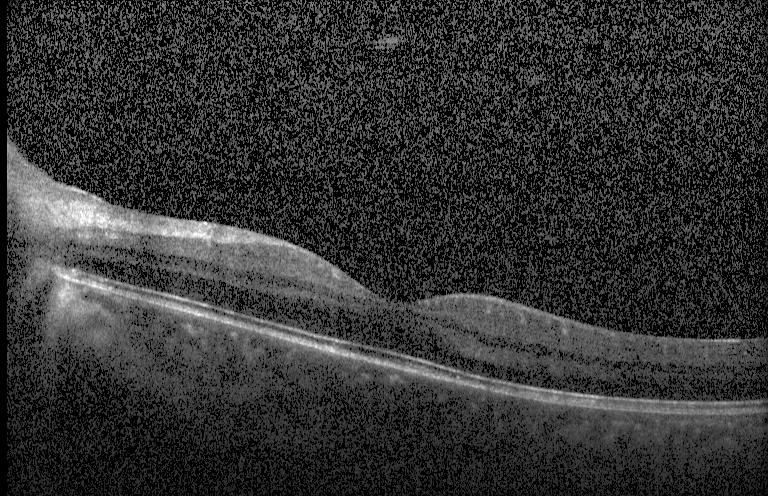

Impression: no evidence of CNV, DME, or drusen.